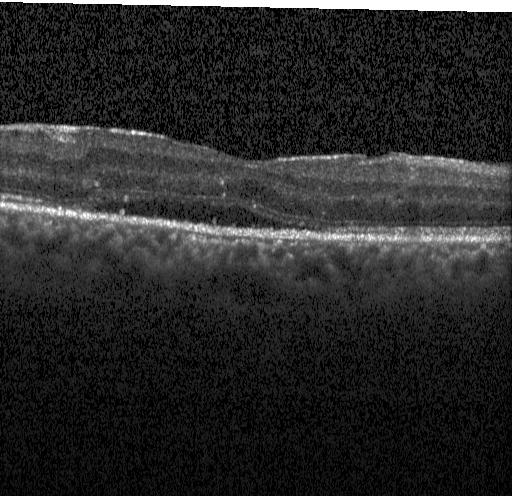
Retinal OCT cross-section — Diagnosis: CNV.